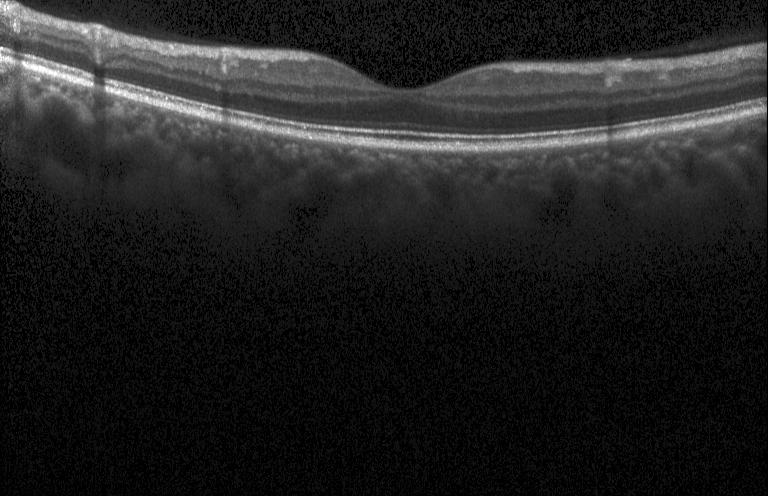
Retinal OCT B-scan, spectral-domain optical coherence tomography, centered on the fovea, Heidelberg Spectralis
Dx: no CNV, DME, or drusen.